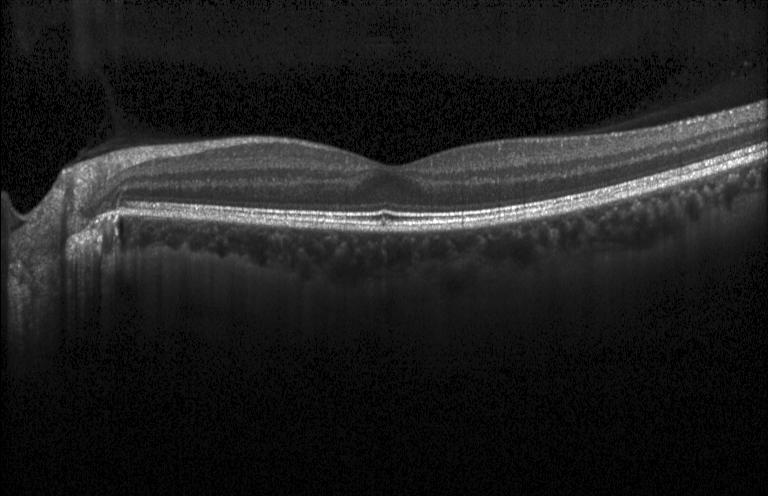
Retinal OCT B-scan. Through the macula — Diagnosis: no CNV, no DME, and no drusen.